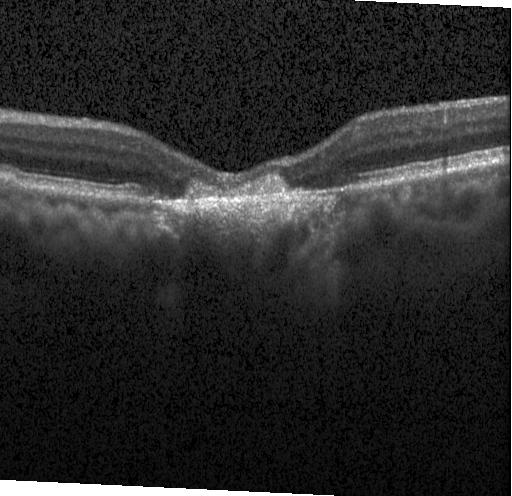

Acquired on a Heidelberg Spectralis. Retinal OCT cross-section. Impression: a choroidal neovascular membrane.